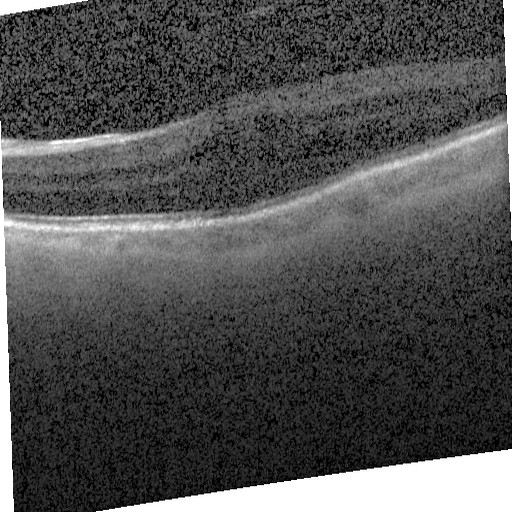 SD-OCT, optical coherence tomography B-scan.
Diagnosis: diabetic macular edema.